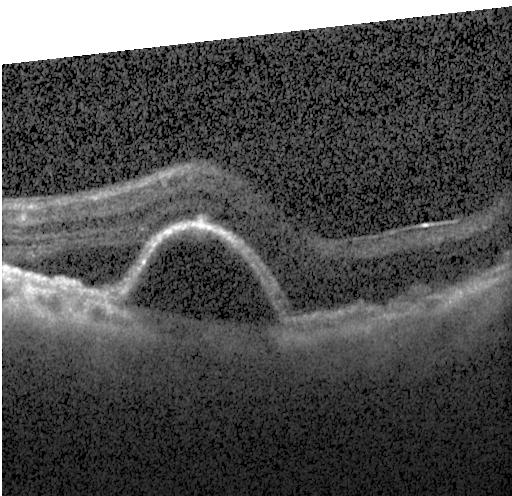

OCT line scan, centered on the fovea, Heidelberg Spectralis, spectral-domain optical coherence tomography. Macular OCT: CNV.